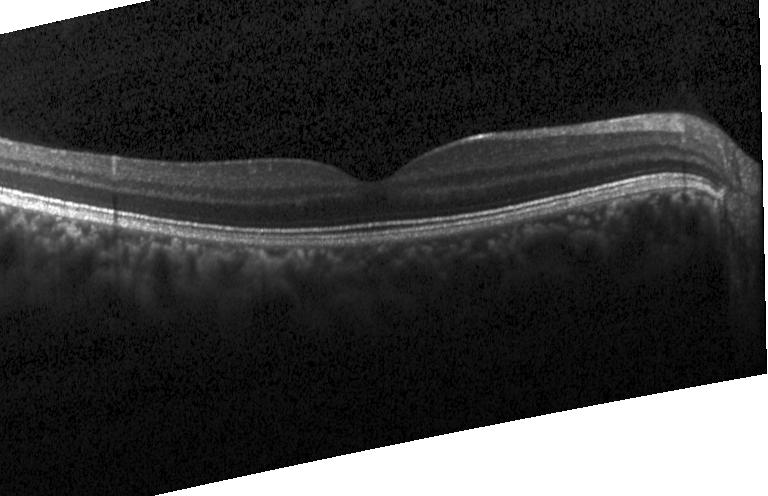
Spectral-domain OCT B-scan: no CNV, no DME, and no drusen.